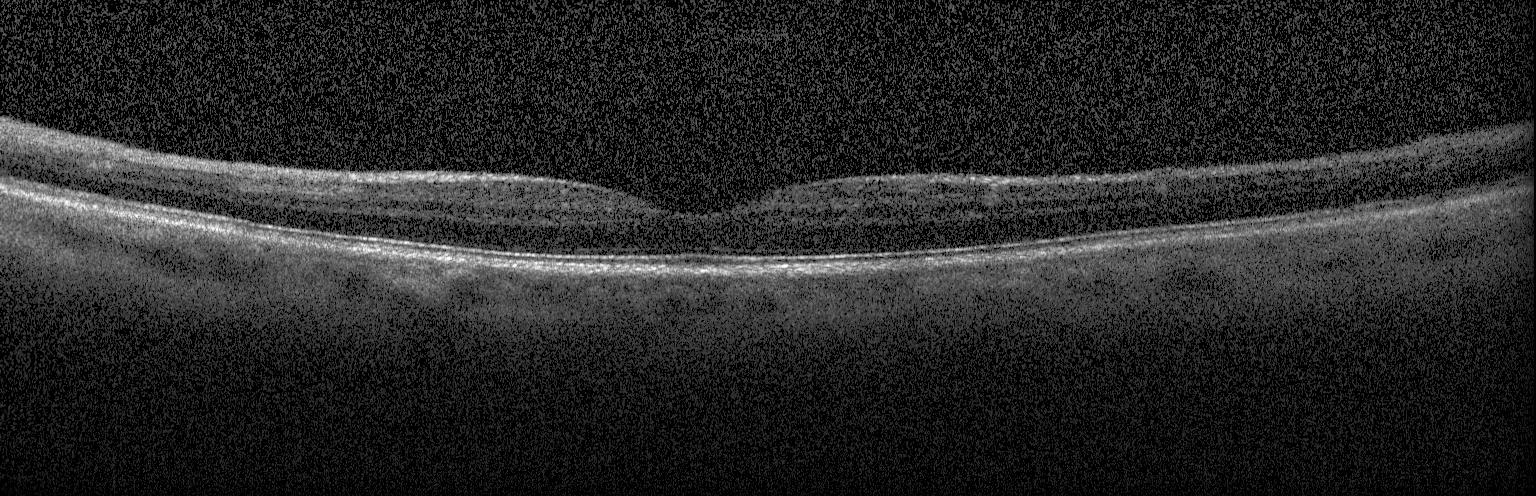

Optical coherence tomography scan.
Impression: no choroidal neovascularization, diabetic macular edema, or drusen.